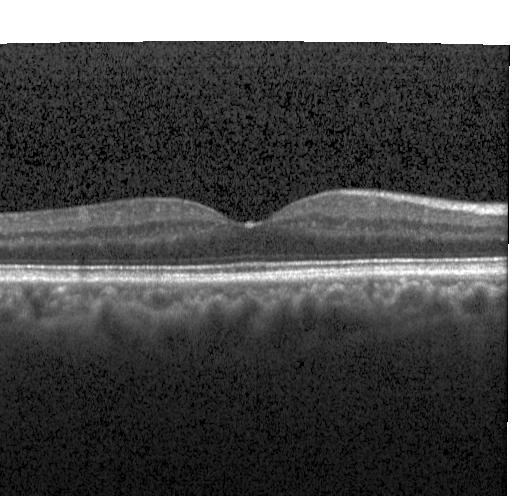
SD-OCT, fovea-centered, retinal OCT cross-section
Finding: neither CNV, DME, nor drusen.